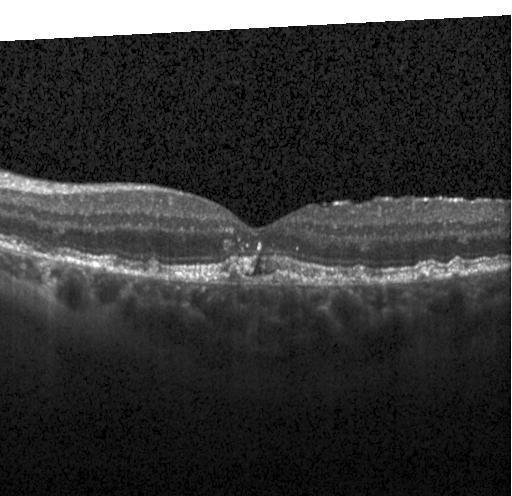

Impression: a choroidal neovascular membrane.